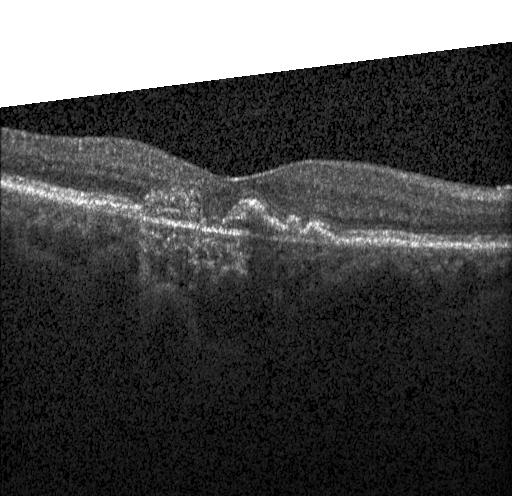

Heidelberg Spectralis OCT system, OCT line scan, SD-OCT
Finding: a choroidal neovascular membrane.